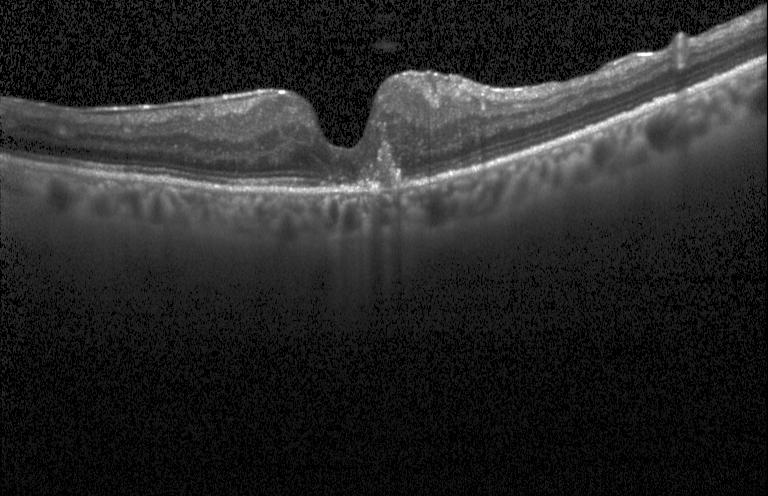 SD-OCT · optical coherence tomography scan · centered on the fovea.
Impression: choroidal neovascularization (CNV).